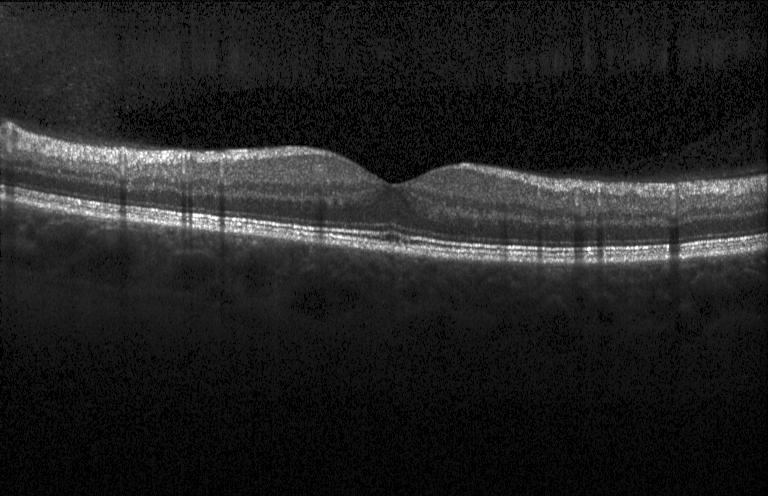
OCT scan showing no choroidal neovascularization, no diabetic macular edema, and no drusen.